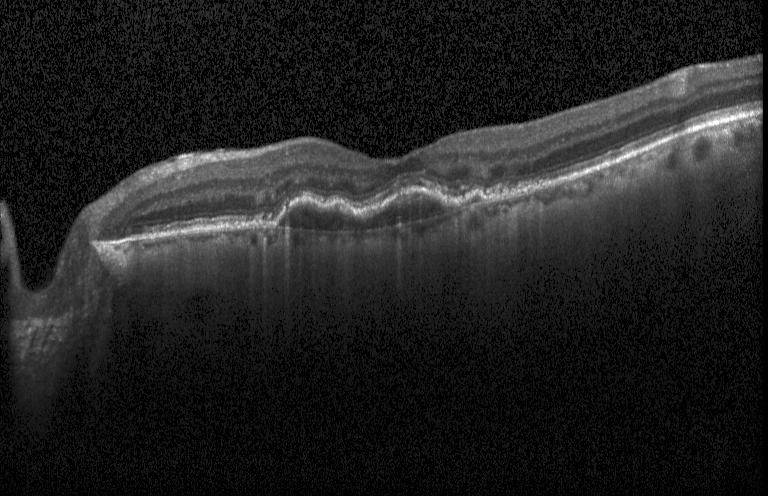

Dx: choroidal neovascularization.